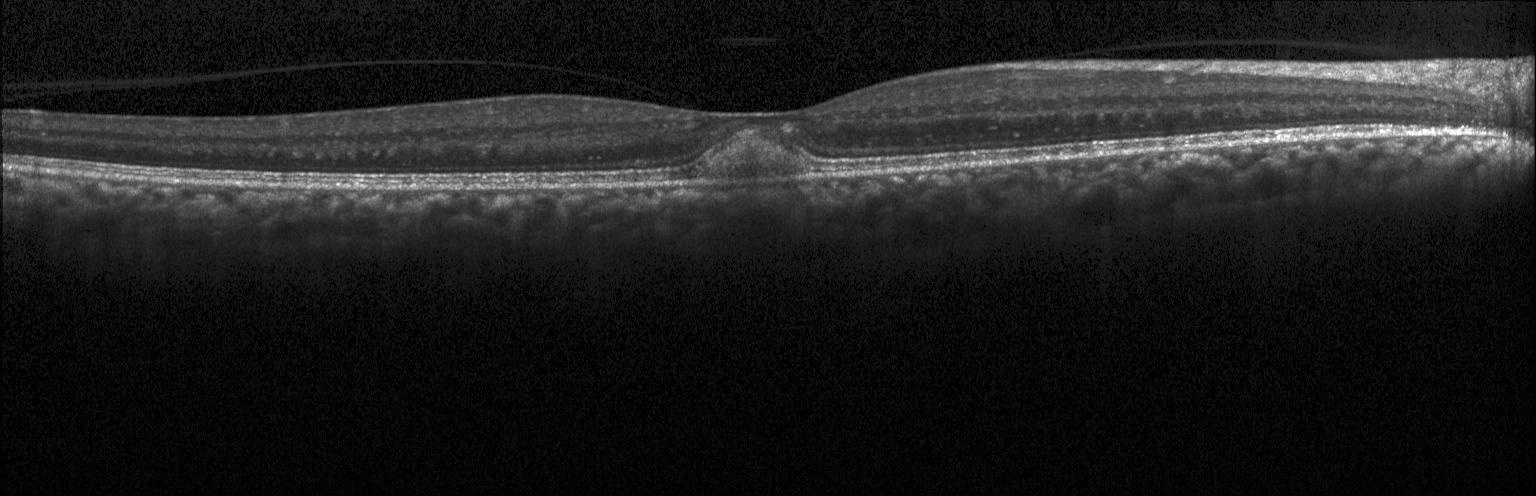

Diagnosis: a choroidal neovascular membrane.